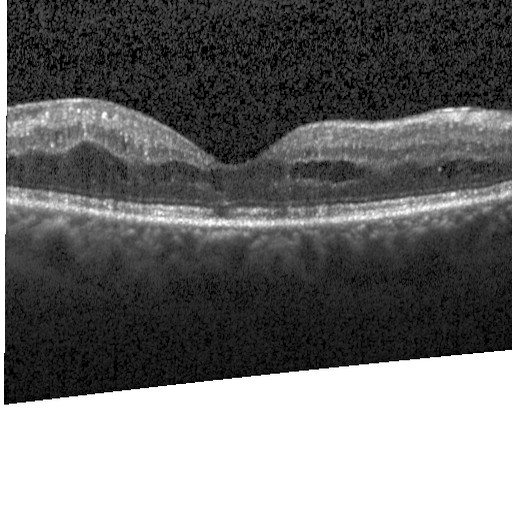

Fovea-centered · spectral-domain optical coherence tomography · acquired on a Heidelberg Spectralis · optical coherence tomography scan. This B-scan demonstrates diabetic macular edema.